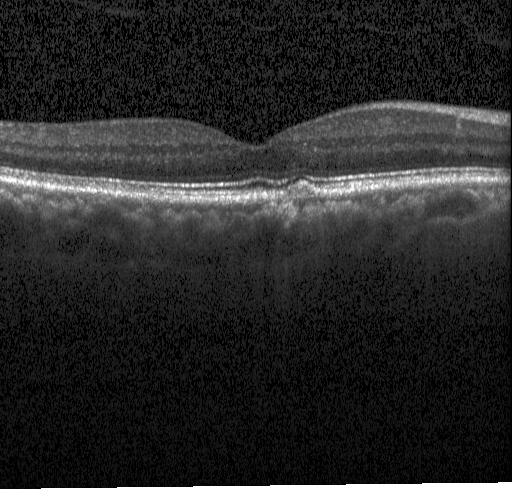
OCT finding: sub-RPE drusenoid deposits.